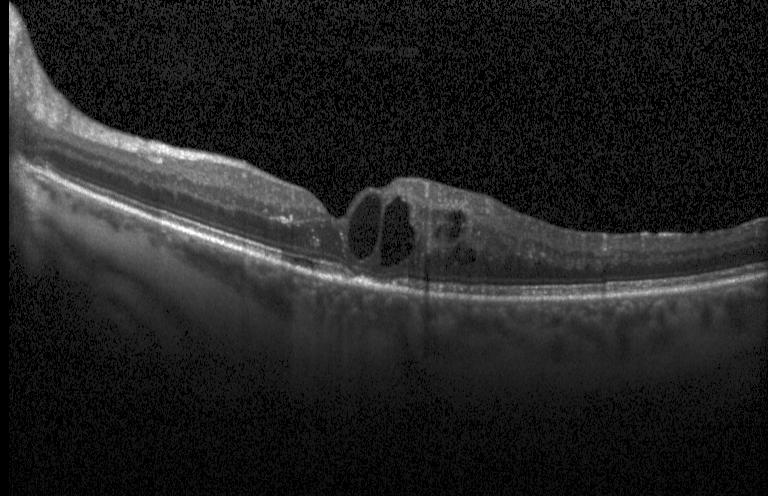
Spectral-domain optical coherence tomography. Macular scan. Heidelberg Spectralis OCT system. OCT line scan.
Diagnosis: DME.